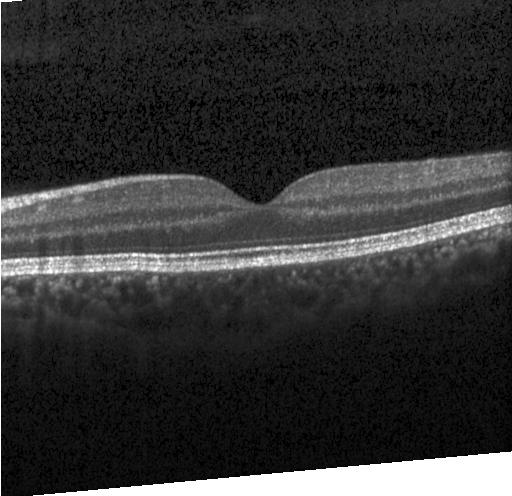 OCT finding: no evidence of choroidal neovascularization, diabetic macular edema, or drusen.